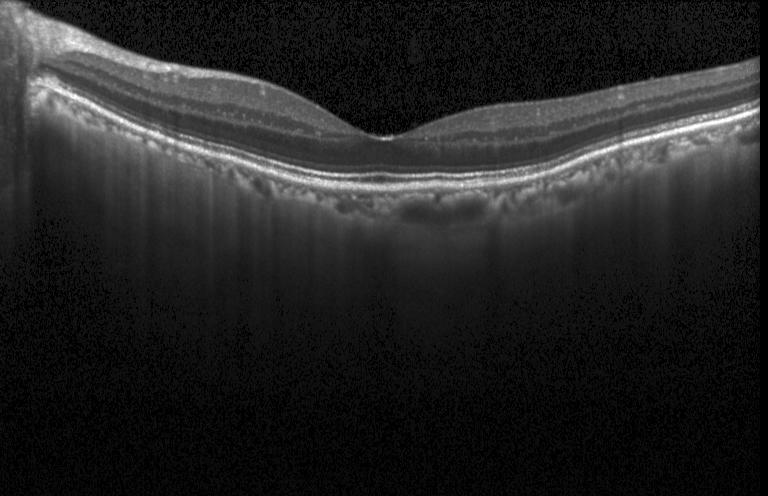

The scan shows no CNV, DME, or drusen.